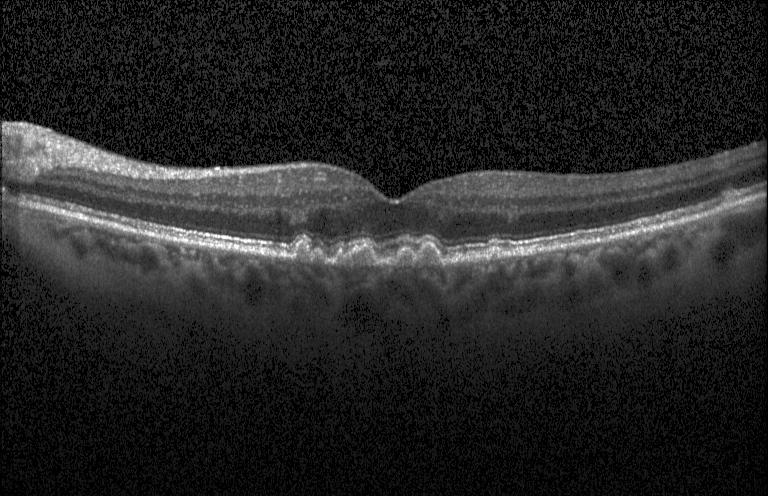
Optical coherence tomography scan — This B-scan demonstrates drusen.